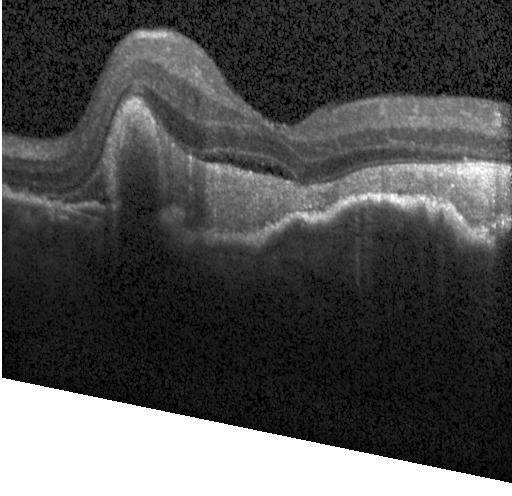 Instrument: Heidelberg Spectralis; optical coherence tomography B-scan
This B-scan demonstrates CNV.